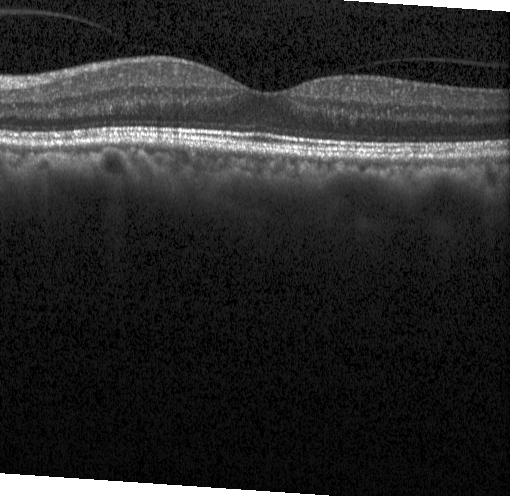

Optical coherence tomography scan
Dx: no choroidal neovascularization, no diabetic macular edema, and no drusen.